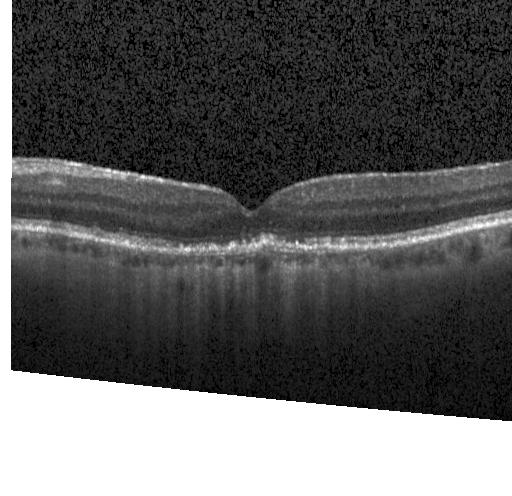

Finding: multiple drusen.